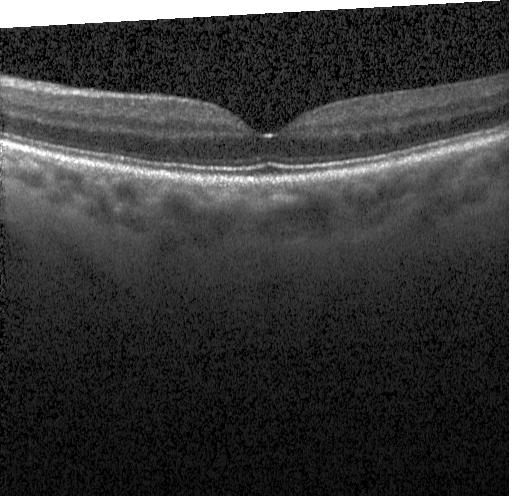

OCT line scan. Acquired on a Heidelberg Spectralis. OCT finding: neither choroidal neovascularization, diabetic macular edema, nor drusen.